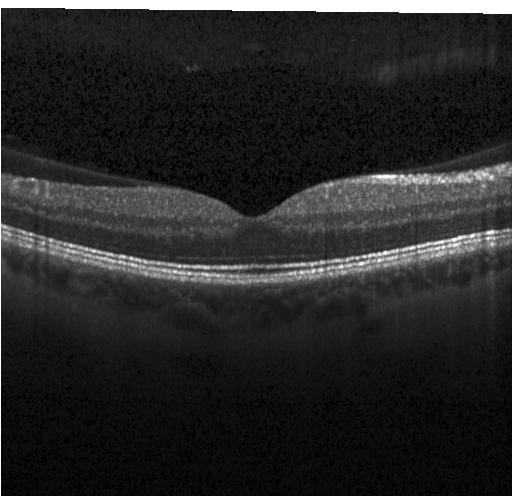

Spectral-domain OCT · optical coherence tomography scan. The scan shows no evidence of CNV, DME, or drusen.